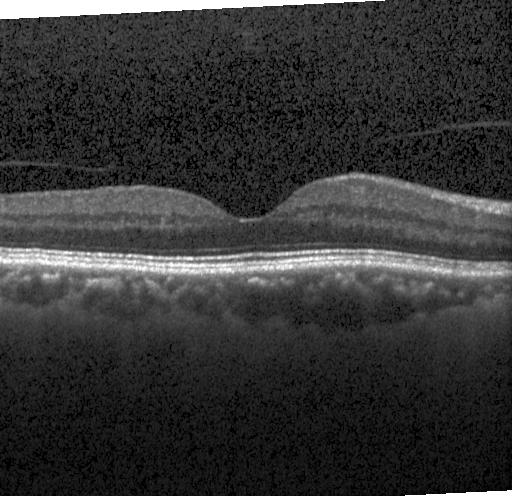 Optical coherence tomography scan, Heidelberg Spectralis OCT system. OCT finding: neither CNV, DME, nor drusen.